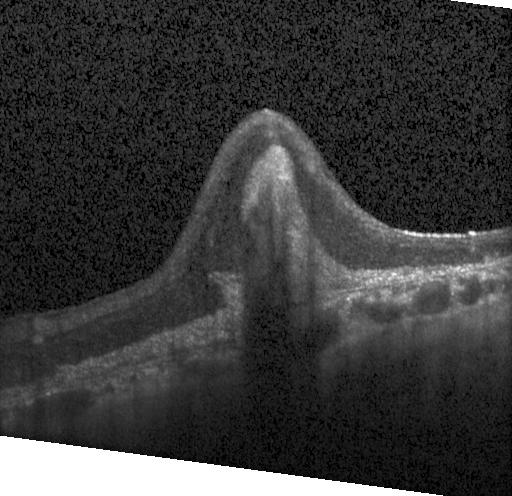 Centered on the fovea. Spectral-domain optical coherence tomography. OCT line scan
Impression: CNV.